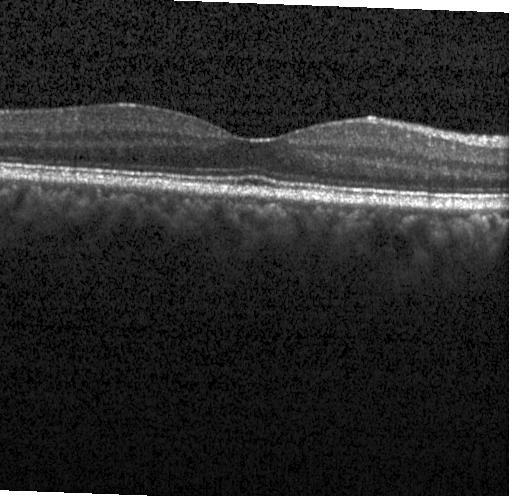

Fovea-centered. Retinal OCT cross-section. Heidelberg Spectralis.
This B-scan demonstrates no CNV, DME, or drusen.